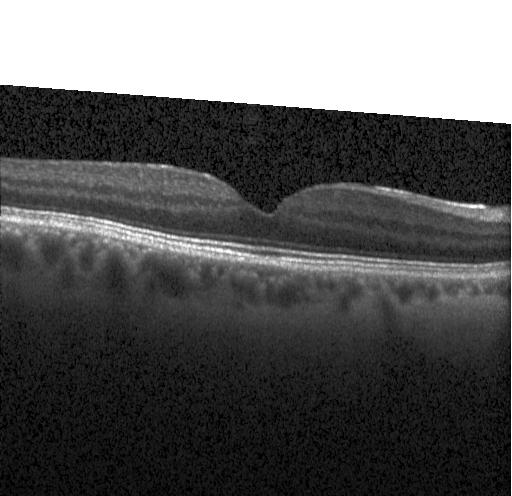

SD-OCT · OCT line scan · macular scan · Heidelberg Spectralis OCT system — Finding: no evidence of CNV, DME, or drusen.